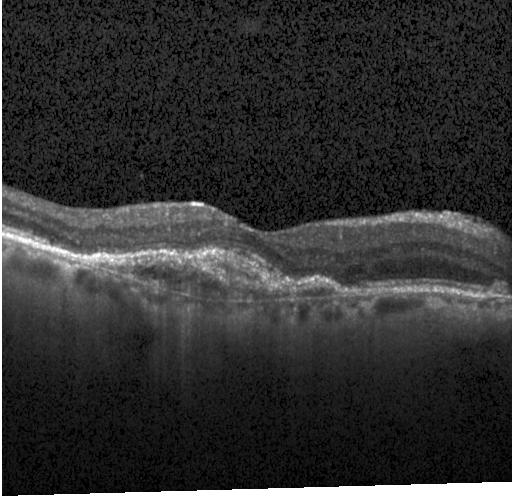 This B-scan demonstrates choroidal neovascularization (CNV).